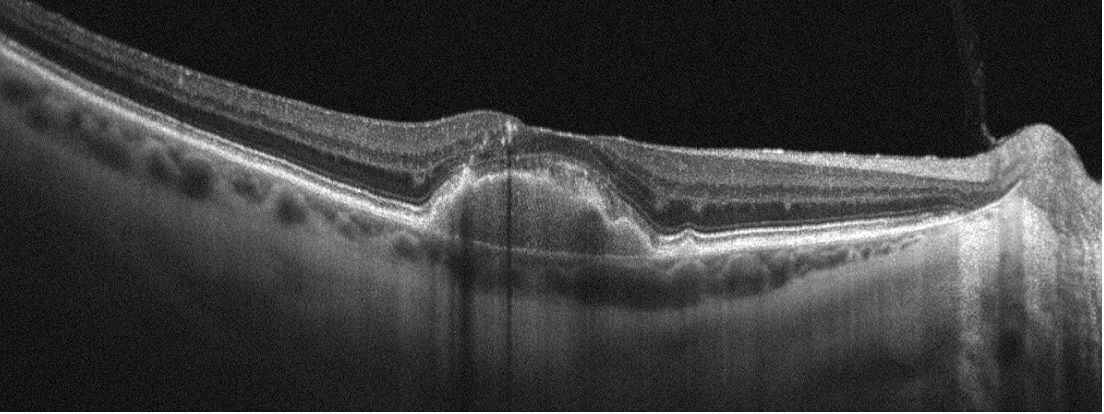

Diagnosis: age-related macular degeneration (AMD).